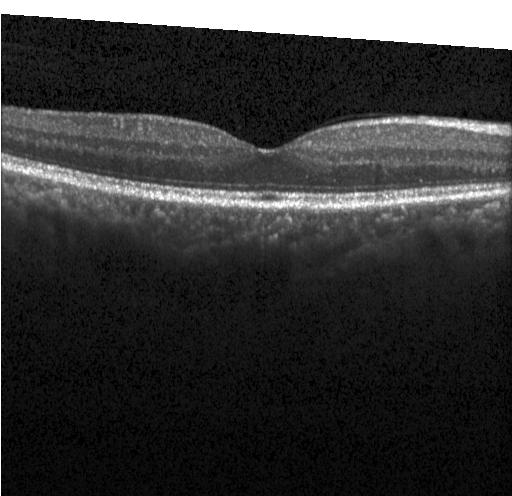
Spectral-domain OCT B-scan: neither choroidal neovascularization, diabetic macular edema, nor drusen.